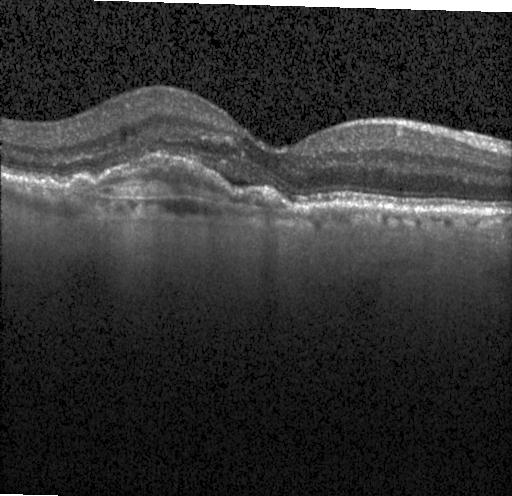
OCT B-scan · horizontal scan through the fovea · spectral-domain OCT.
Finding: choroidal neovascularization (CNV).